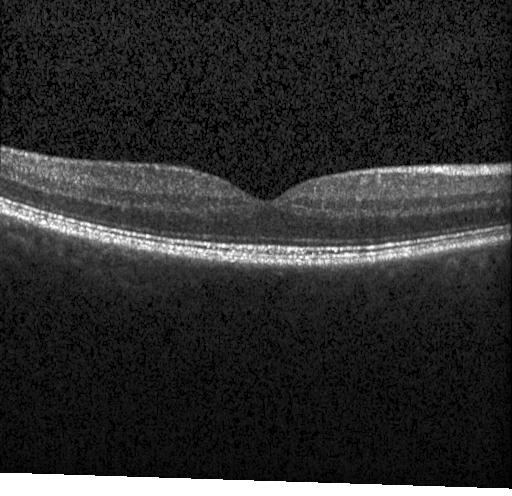

Dx: no evidence of choroidal neovascularization, diabetic macular edema, or drusen.